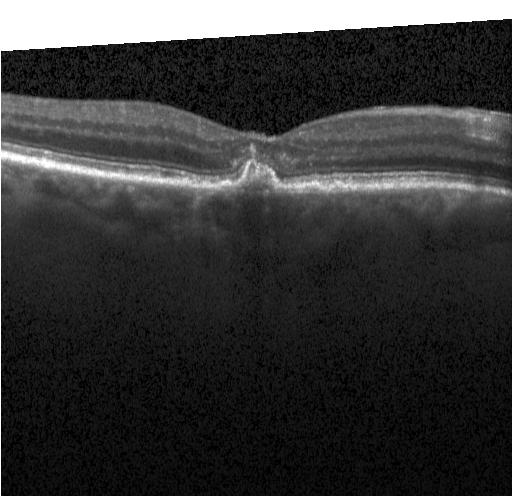

Impression: a choroidal neovascular membrane.